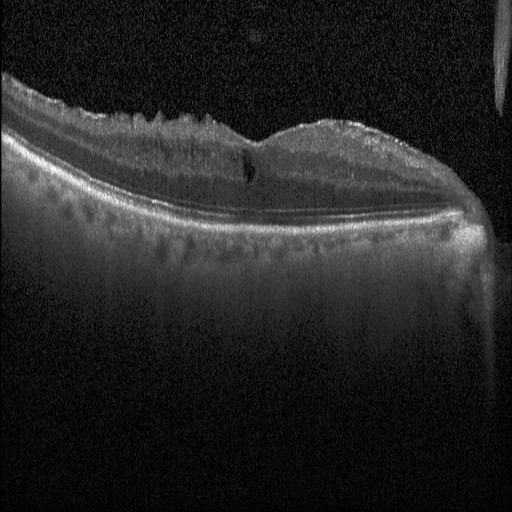

OCT B-scan. Spectral-domain optical coherence tomography. Macular scan.
Finding: diabetic macular edema.